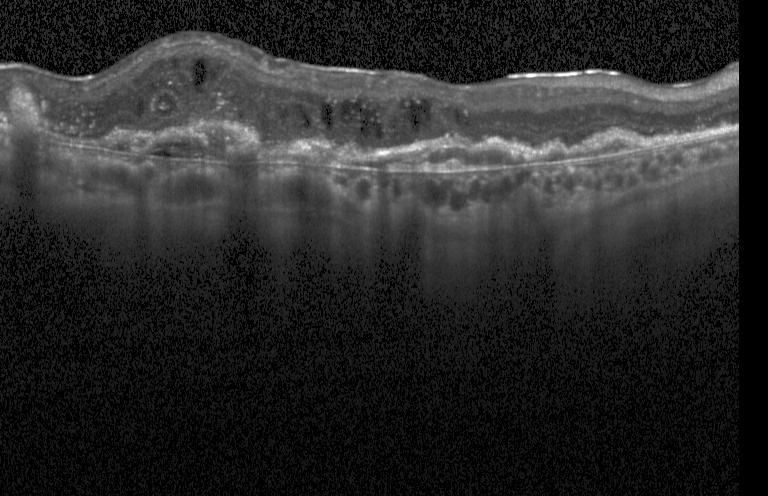

Through the macula. Acquired on a Heidelberg Spectralis. OCT line scan. Impression: a choroidal neovascular membrane.